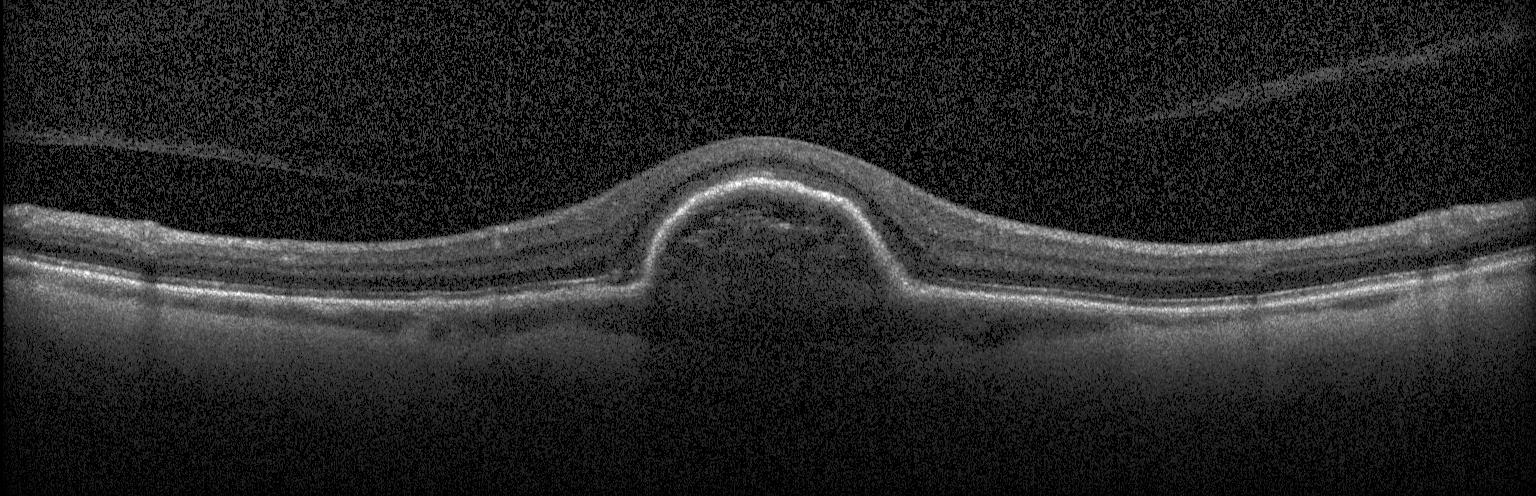

Retinal OCT cross-section · horizontal scan through the fovea — Finding: a choroidal neovascular membrane.